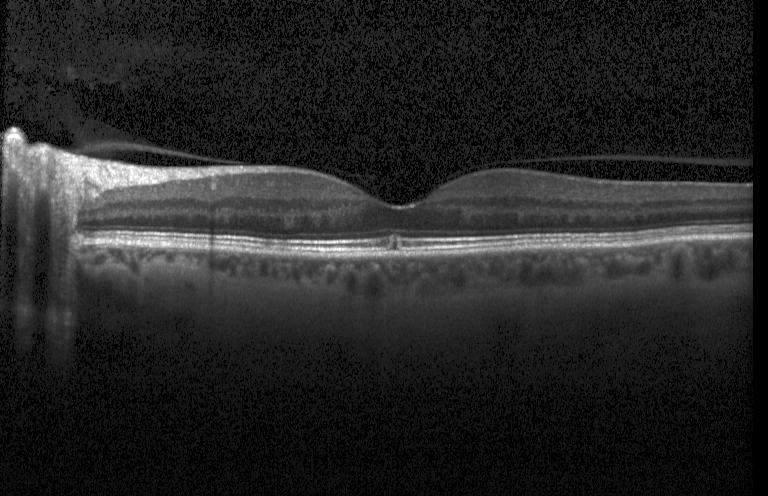
Horizontal scan through the fovea, optical coherence tomography scan. Impression: no choroidal neovascularization, diabetic macular edema, or drusen.